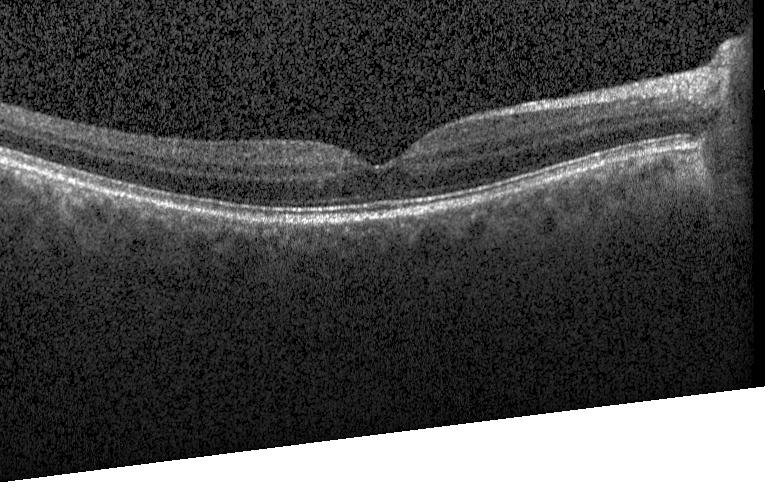 Instrument: Heidelberg Spectralis, OCT line scan
Assessment: neither choroidal neovascularization, diabetic macular edema, nor drusen.